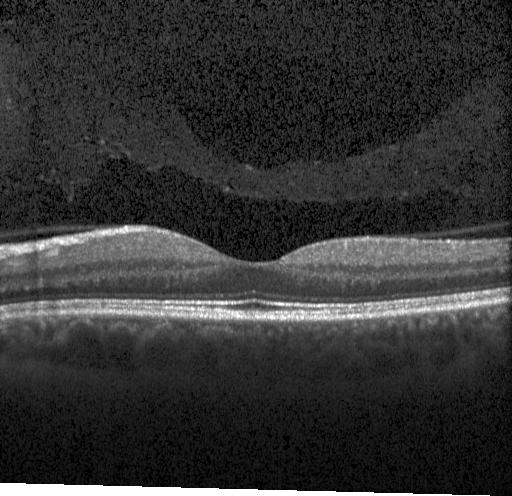 Dx: no choroidal neovascularization, diabetic macular edema, or drusen.